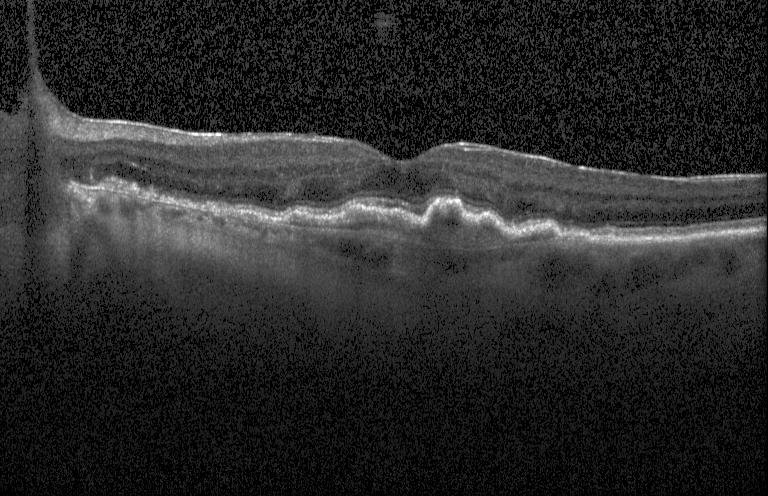 Heidelberg Spectralis · through the macula · OCT B-scan — Diagnosis: a choroidal neovascular membrane.